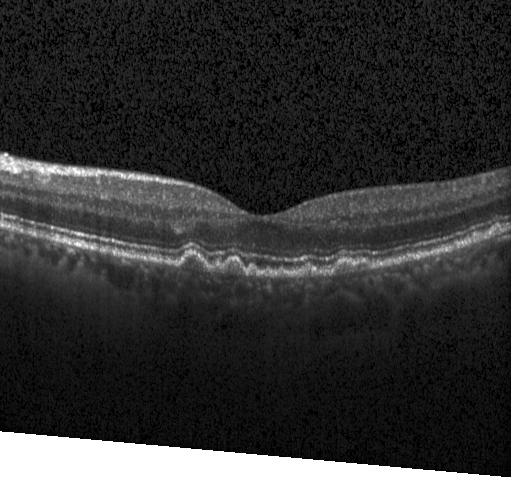 Impression: multiple drusen.